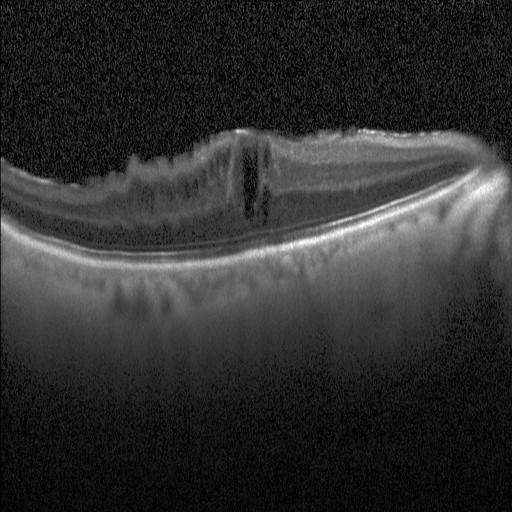 Diagnosis: DME.